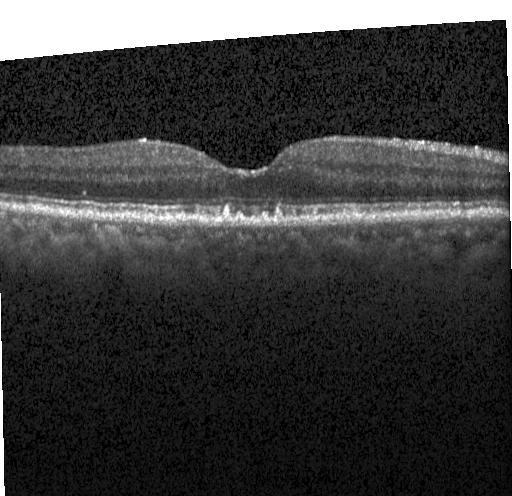

Heidelberg Spectralis. Optical coherence tomography scan.
Macular OCT: drusen.